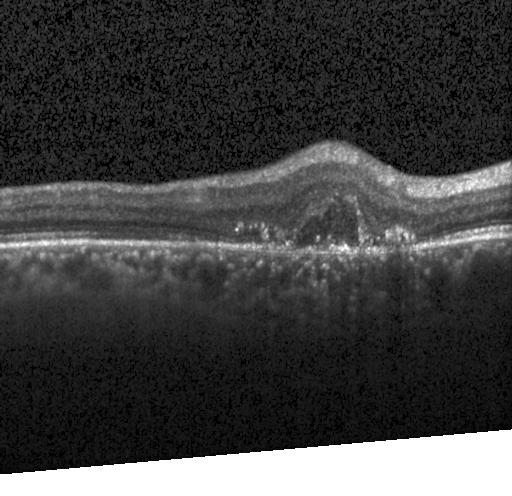
Impression: a choroidal neovascular membrane.